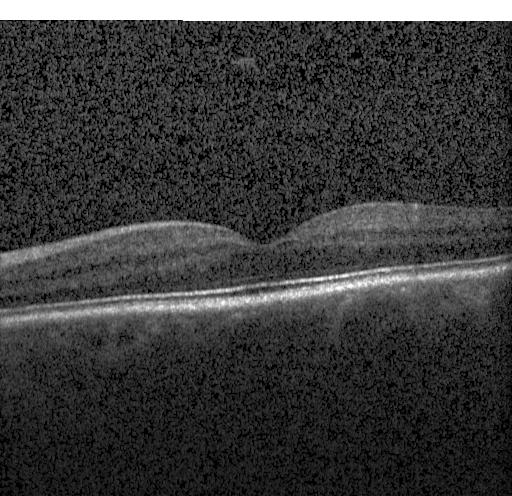

The scan shows neither choroidal neovascularization, diabetic macular edema, nor drusen.